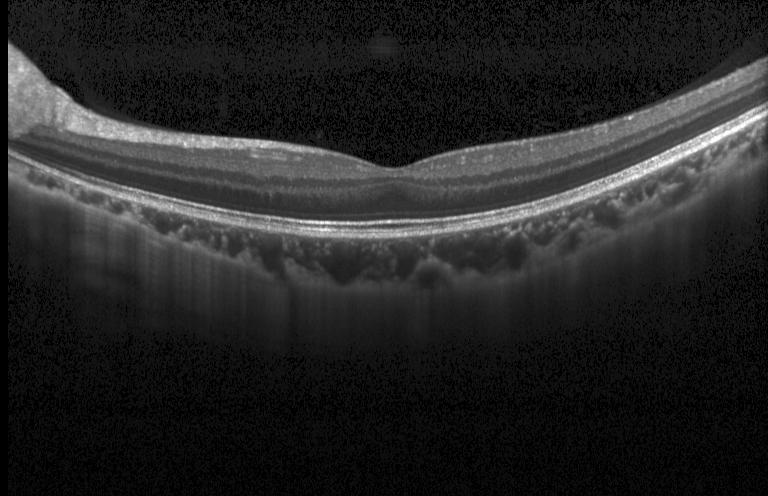

OCT line scan. SD-OCT. Through the macula. Instrument: Heidelberg Spectralis.
Impression: no evidence of choroidal neovascularization, diabetic macular edema, or drusen.